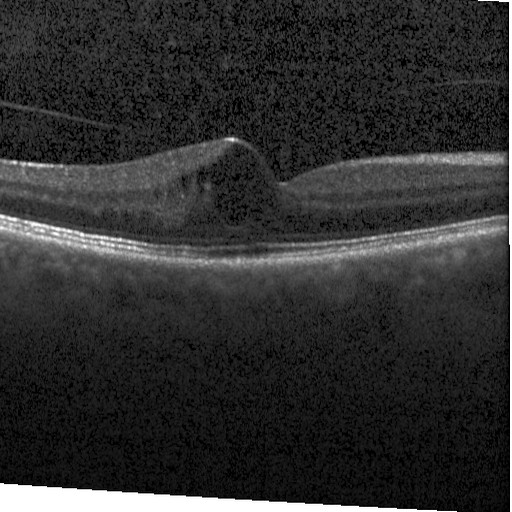 Spectral-domain OCT; optical coherence tomography B-scan. Dx: DME.